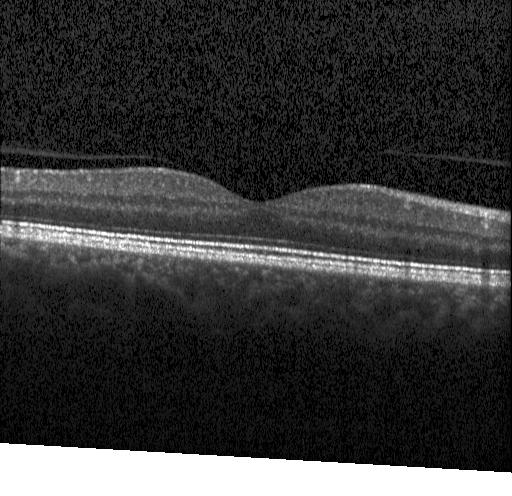 OCT B-scan
Dx: neither choroidal neovascularization, diabetic macular edema, nor drusen.